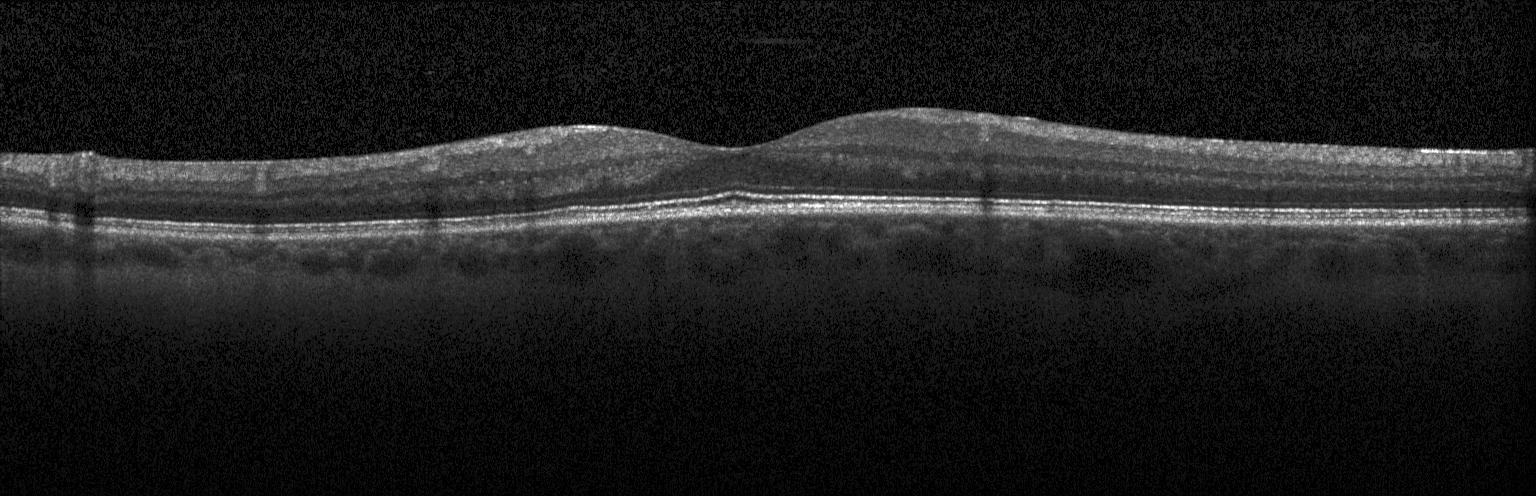
Retinal OCT B-scan; instrument: Heidelberg Spectralis; horizontal scan through the fovea. This B-scan demonstrates neither choroidal neovascularization, diabetic macular edema, nor drusen.